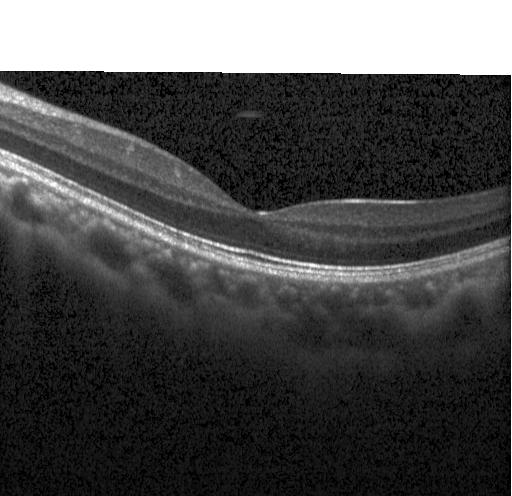

OCT line scan — Finding: no choroidal neovascularization, diabetic macular edema, or drusen.